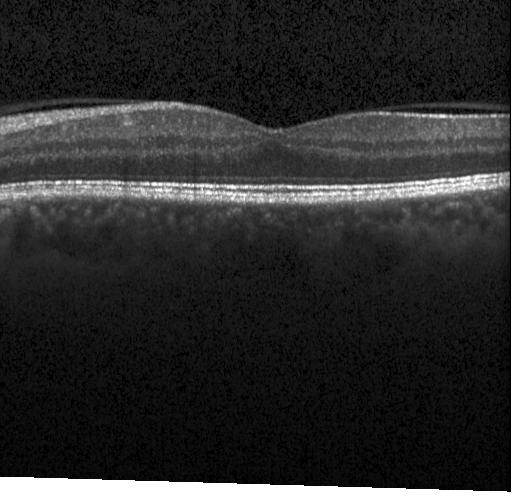

Diagnosis: no choroidal neovascularization, diabetic macular edema, or drusen.